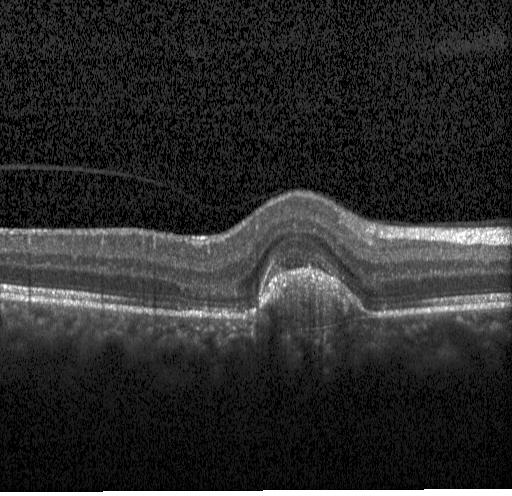
Retinal OCT cross-section showing a choroidal neovascular membrane.